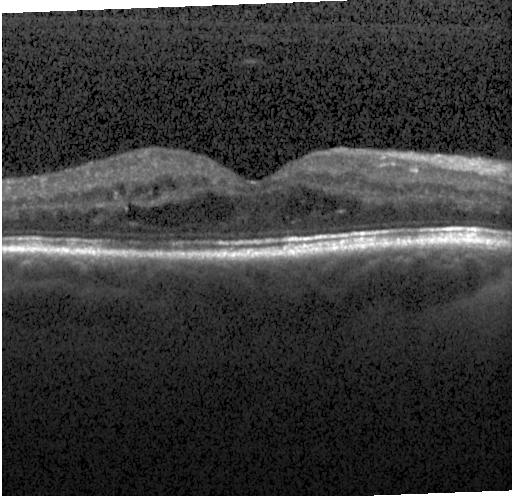

Through the macula. Optical coherence tomography B-scan. Heidelberg Spectralis — Assessment: DME.